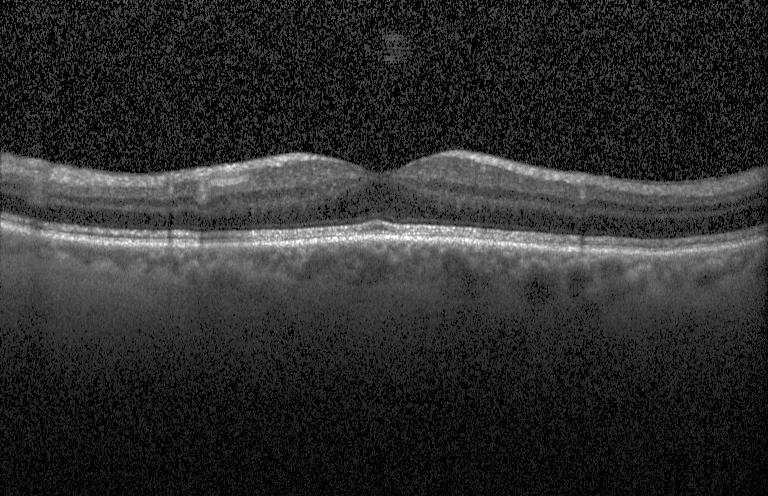

Diagnosis: no CNV, DME, or drusen.